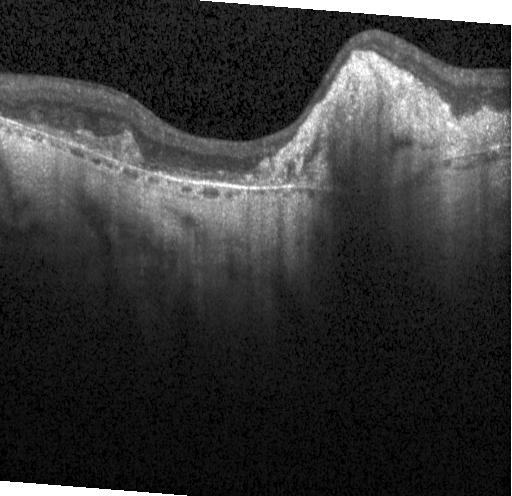

Dx: choroidal neovascularization.